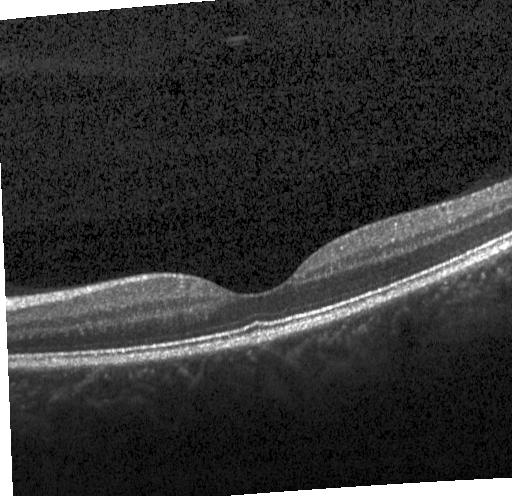

Diagnosis: no choroidal neovascularization, no diabetic macular edema, and no drusen.